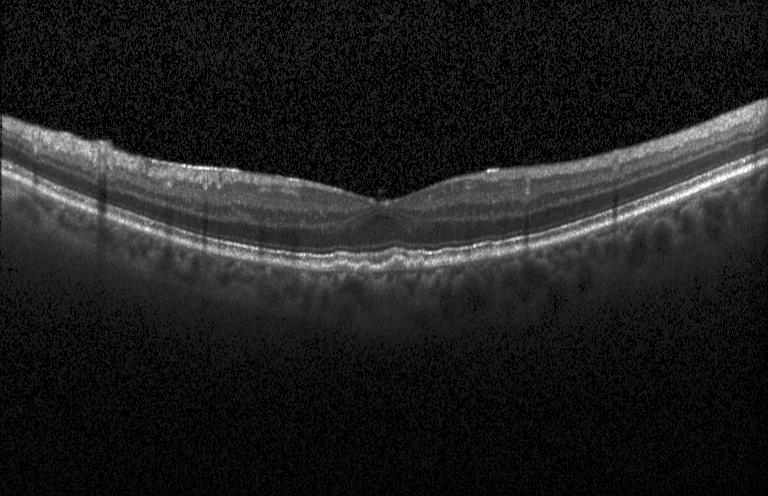 SD-OCT. Optical coherence tomography scan — Impression: sub-RPE drusenoid deposits.